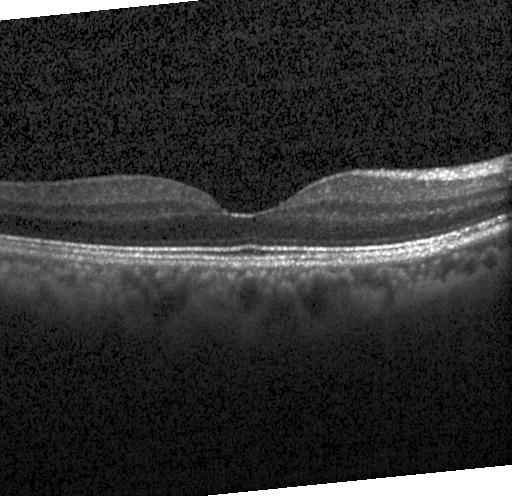 Spectral-domain OCT B-scan: no evidence of choroidal neovascularization, diabetic macular edema, or drusen.